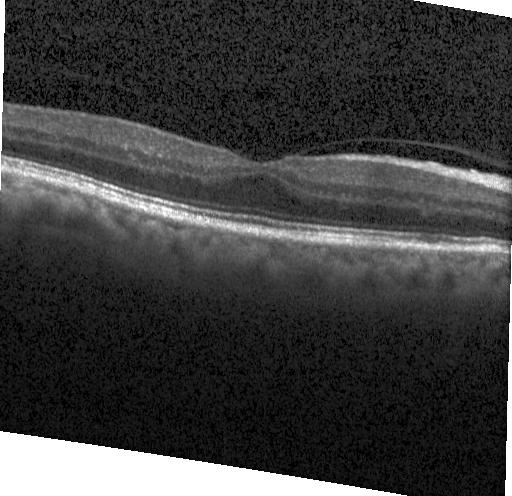
Retinal OCT cross-section — This B-scan demonstrates no evidence of CNV, DME, or drusen.